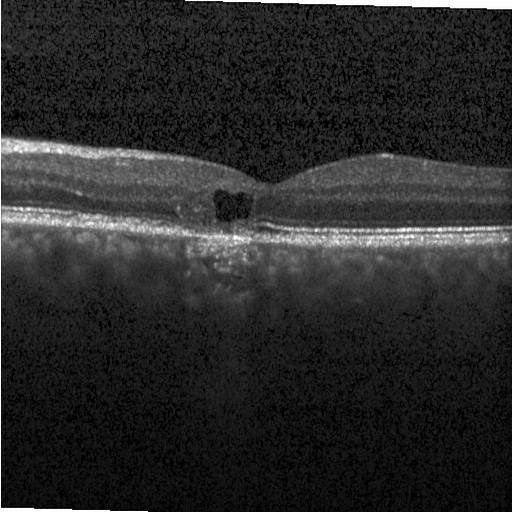
Through the macula; spectral-domain optical coherence tomography; retinal OCT B-scan — Macular OCT: diabetic macular edema.